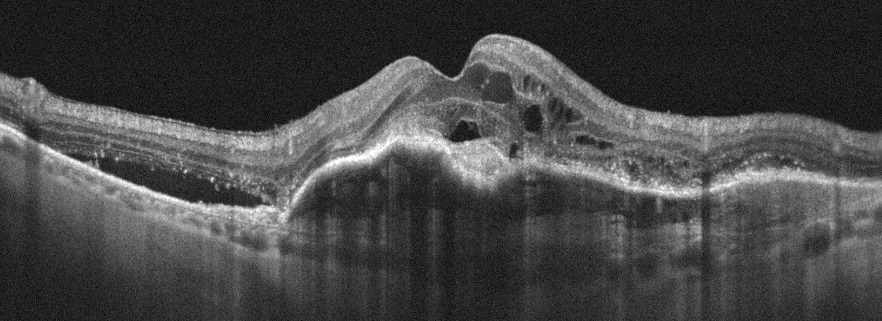

OCT B-scan. Optovue Avanti RTVue XR — Finding: age-related macular degeneration.